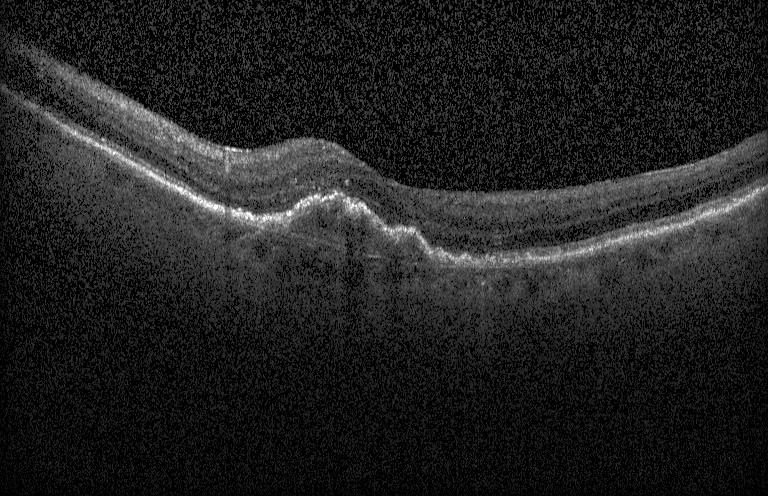 Horizontal scan through the fovea, retinal OCT B-scan, Heidelberg Spectralis — Assessment: CNV.